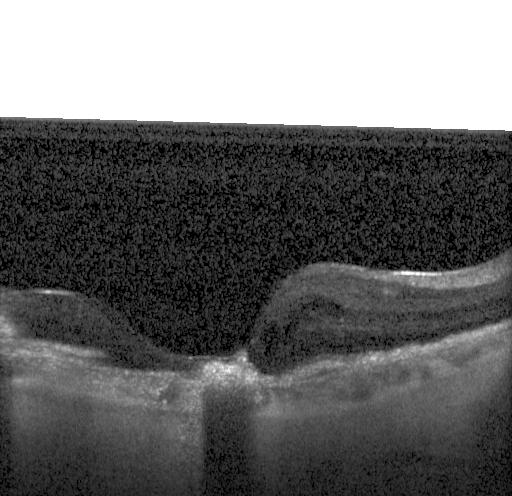 OCT B-scan, through the macula.
Macular OCT: a choroidal neovascular membrane.